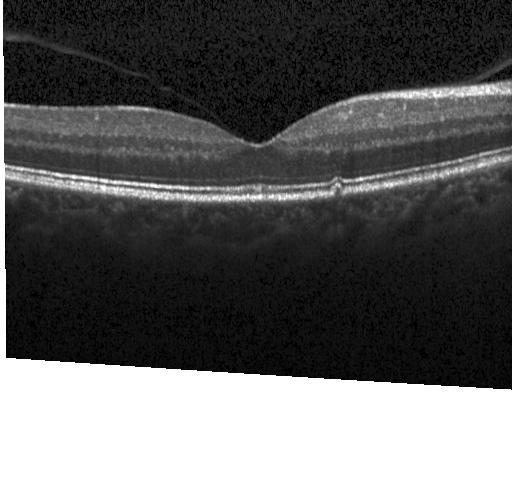
Impression: multiple drusen.